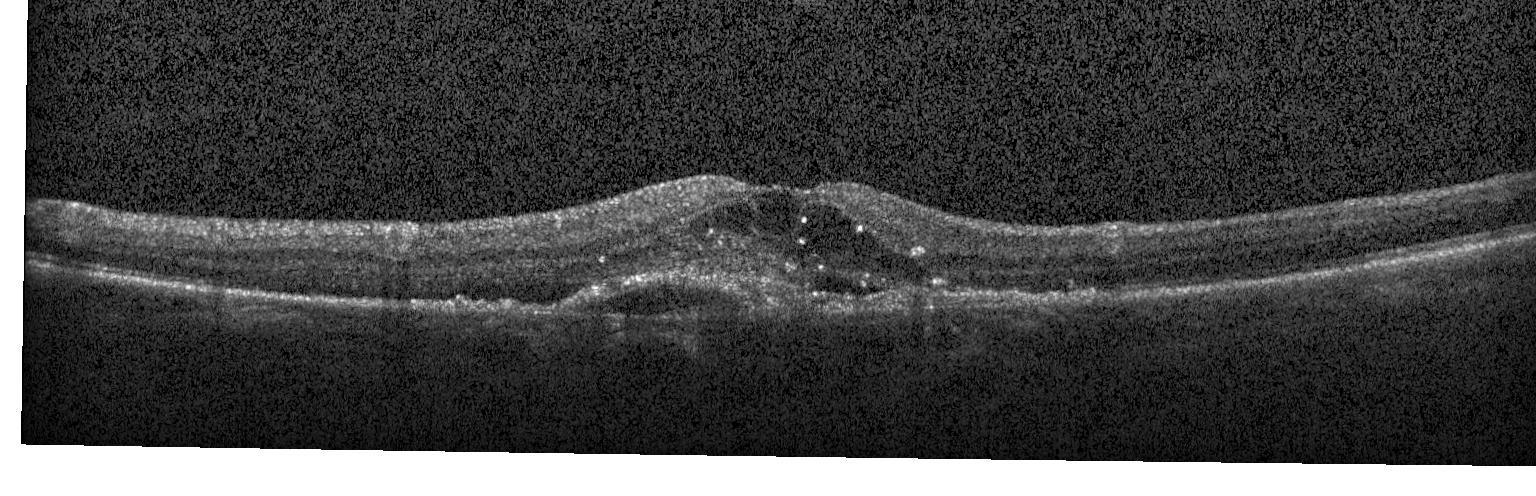 Finding: choroidal neovascularization (CNV).